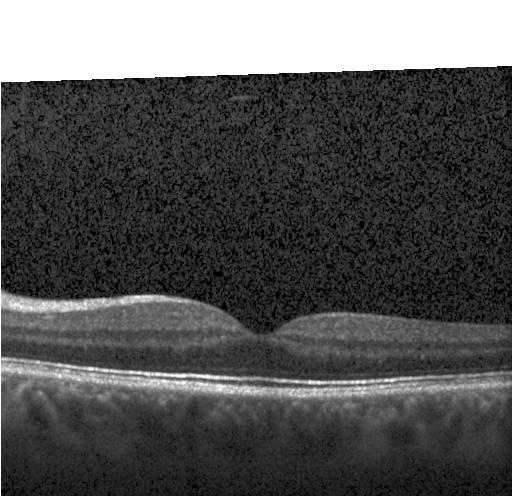

Instrument: Heidelberg Spectralis · spectral-domain OCT · through the macula · retinal OCT cross-section — Finding: no choroidal neovascularization, no diabetic macular edema, and no drusen.